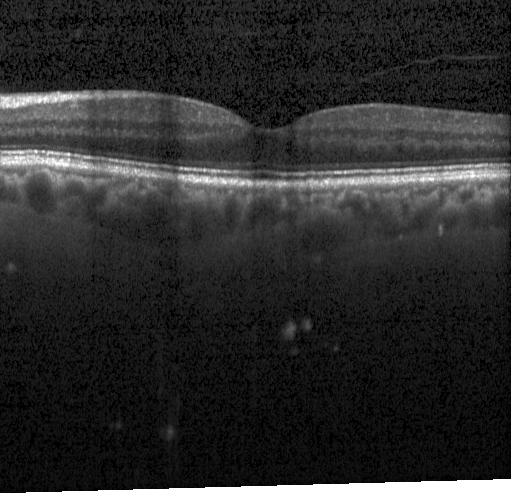
Optical coherence tomography scan
Finding: no choroidal neovascularization, diabetic macular edema, or drusen.